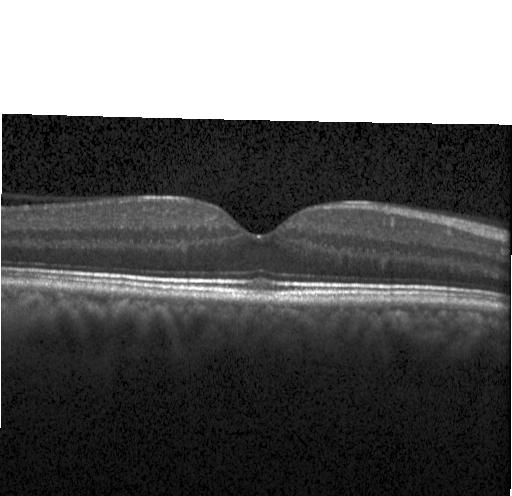 The scan shows no choroidal neovascularization, diabetic macular edema, or drusen.